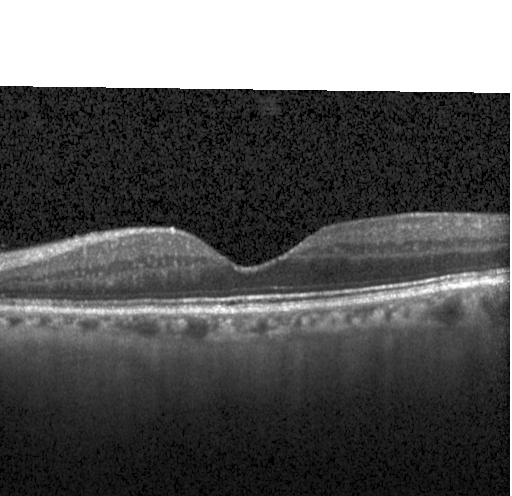
SD-OCT · macular scan · retinal OCT cross-section — This B-scan demonstrates no choroidal neovascularization, no diabetic macular edema, and no drusen.